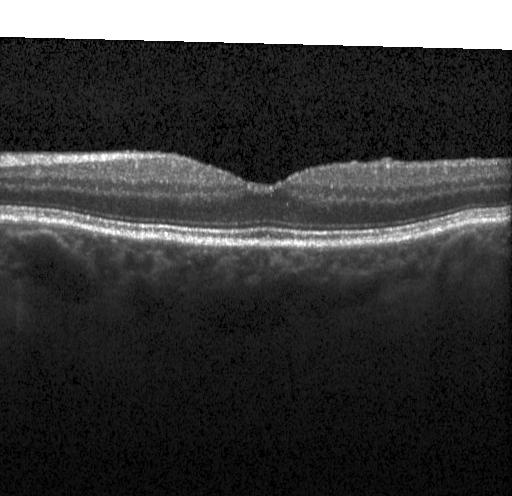 Optical coherence tomography B-scan.
Diagnosis: no evidence of choroidal neovascularization, diabetic macular edema, or drusen.